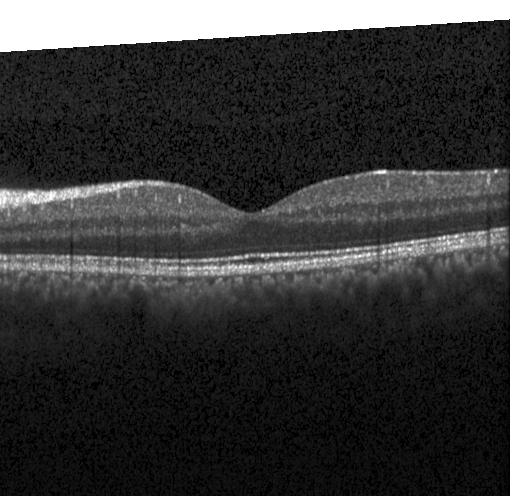

Finding: neither choroidal neovascularization, diabetic macular edema, nor drusen.